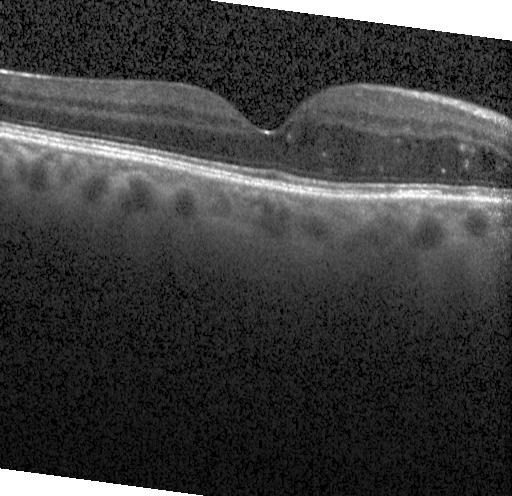 Finding: diabetic macular edema (DME).